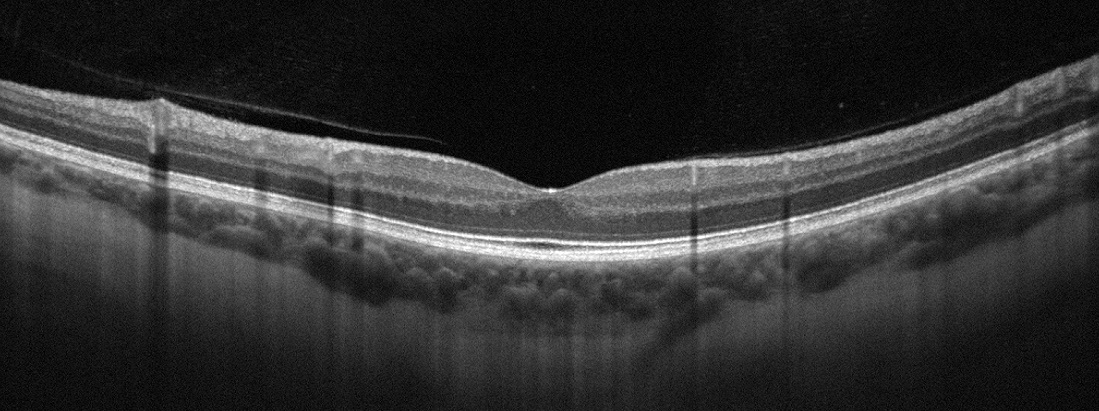
Dx: no evidence of AMD, DME, ERM, RAO, RVO, or VID.